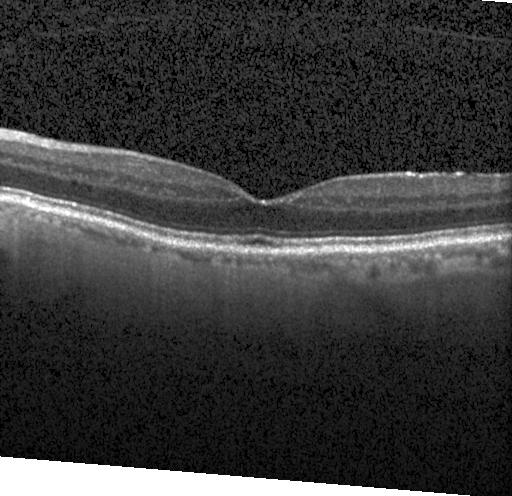

Macular OCT: no evidence of choroidal neovascularization, diabetic macular edema, or drusen.